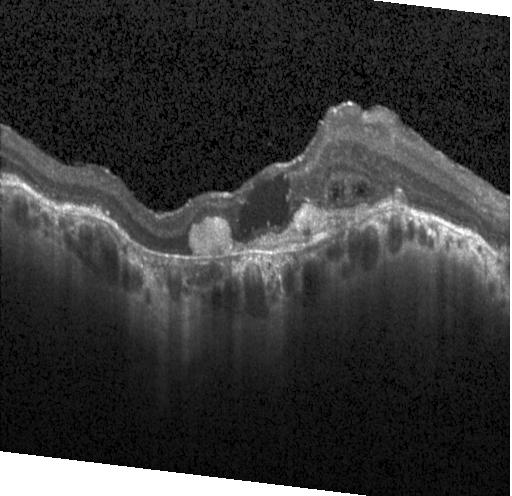
Dx: a choroidal neovascular membrane.